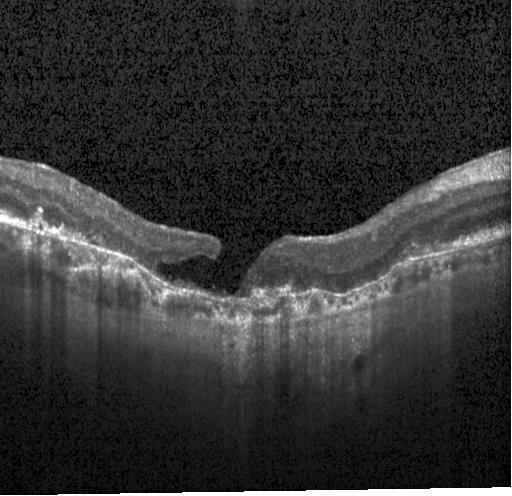

Impression: CNV.